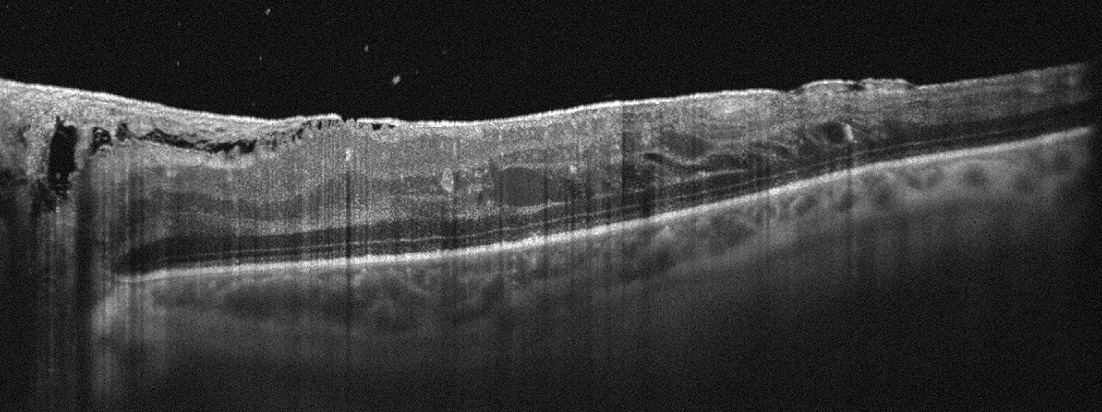 Retinal OCT B-scan, through the macula, acquired on an Optovue Avanti RTVue XR — Diagnosis: diabetic macular edema.